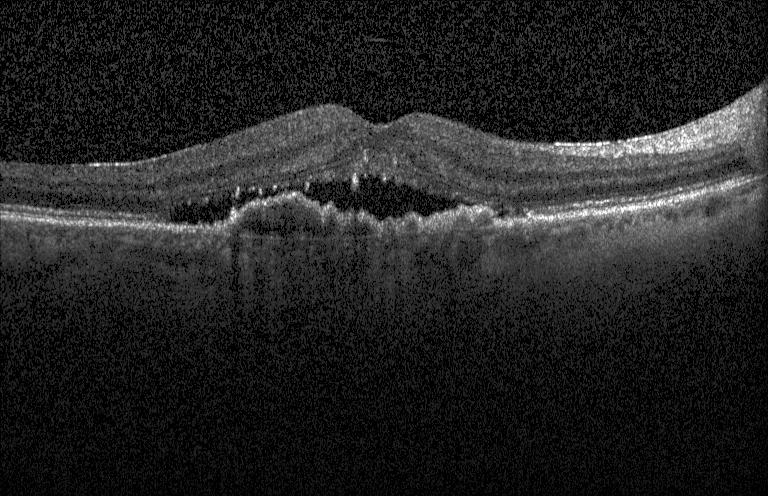 Instrument: Heidelberg Spectralis · spectral-domain OCT · optical coherence tomography scan · macular scan. This B-scan demonstrates choroidal neovascularization (CNV).